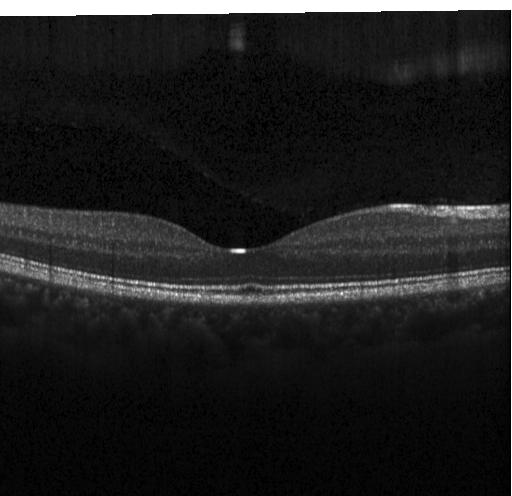

Optical coherence tomography B-scan — OCT finding: neither choroidal neovascularization, diabetic macular edema, nor drusen.